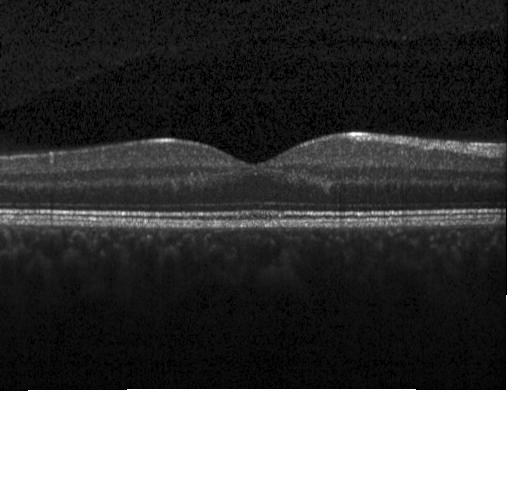
No choroidal neovascularization, diabetic macular edema, or drusen.